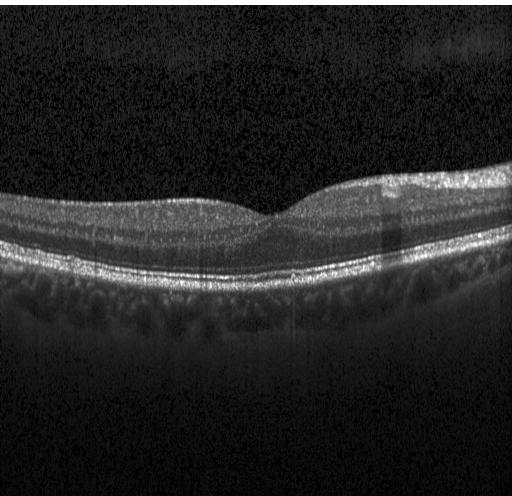 Spectral-domain OCT B-scan: neither choroidal neovascularization, diabetic macular edema, nor drusen.